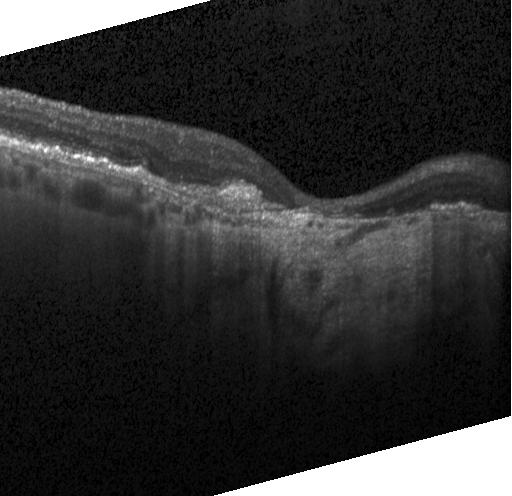 Spectral-domain OCT, Heidelberg Spectralis, optical coherence tomography B-scan, horizontal scan through the fovea — A choroidal neovascular membrane.